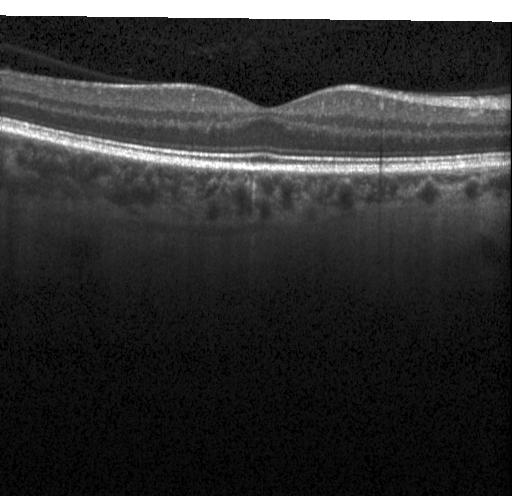

Optical coherence tomography scan; spectral-domain optical coherence tomography; Heidelberg Spectralis OCT system — OCT finding: no choroidal neovascularization, diabetic macular edema, or drusen.